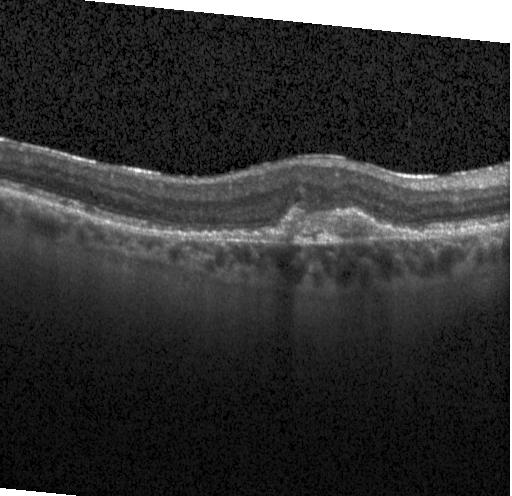

Retinal OCT cross-section; macular scan; spectral-domain optical coherence tomography. The scan shows a choroidal neovascular membrane.